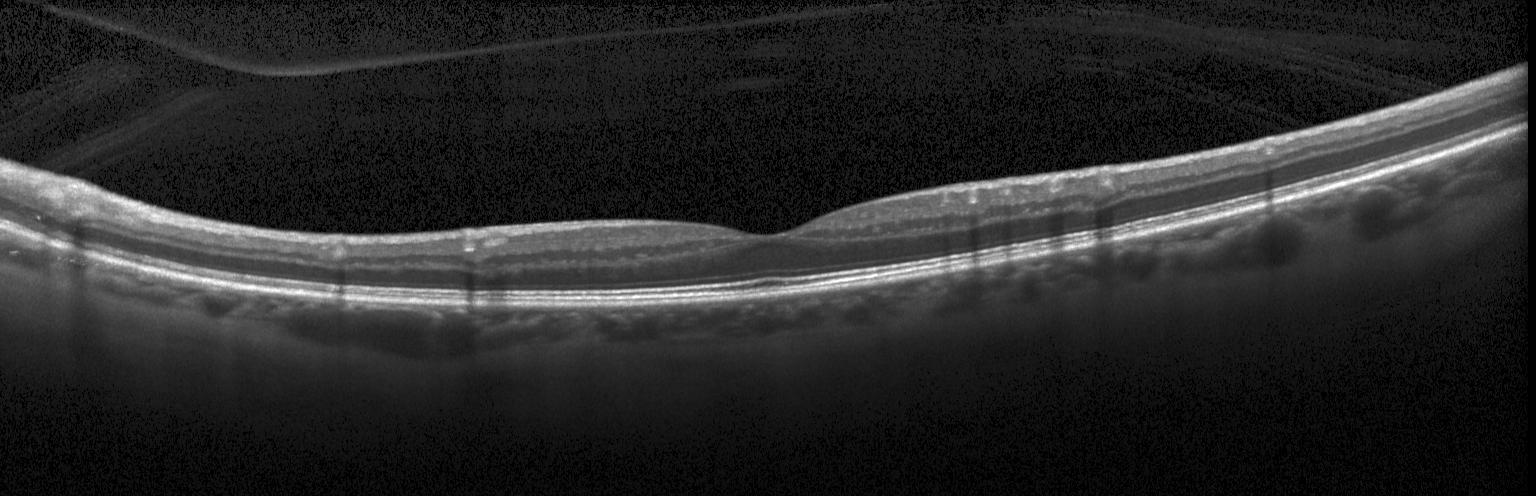

Retinal OCT B-scan.
This B-scan demonstrates no CNV, DME, or drusen.